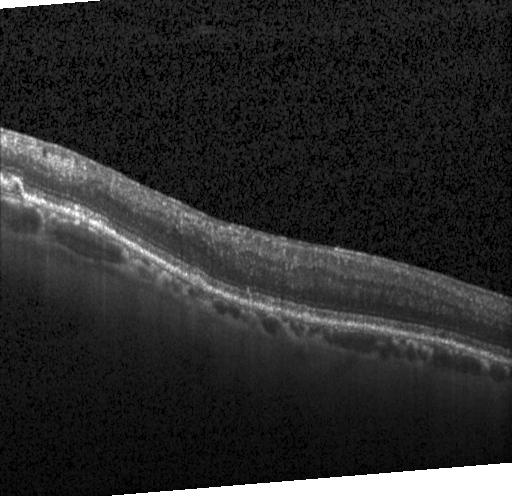 Spectral-domain optical coherence tomography · retinal OCT B-scan.
Finding: a choroidal neovascular membrane.